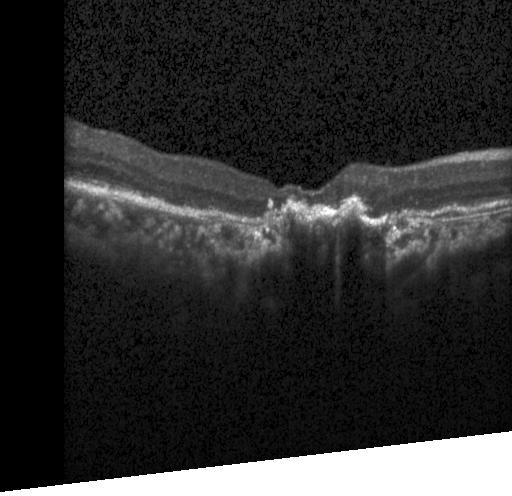 Through the macula, instrument: Heidelberg Spectralis, SD-OCT, OCT line scan.
Diagnosis: CNV.